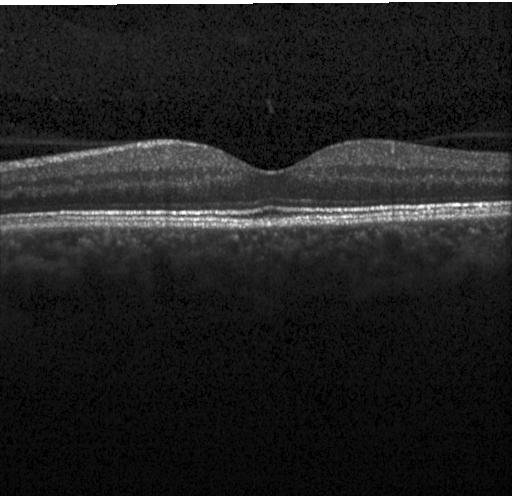

Finding: no choroidal neovascularization, no diabetic macular edema, and no drusen.